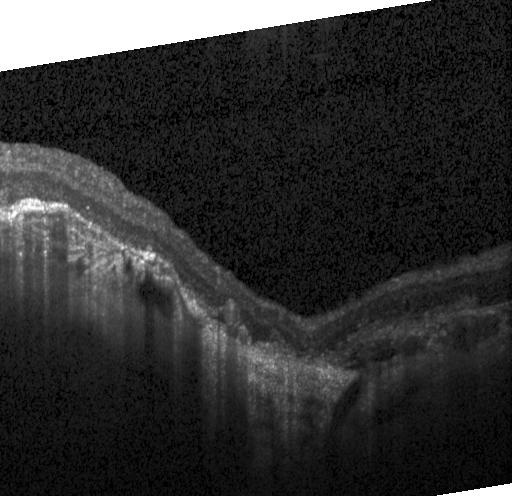
Optical coherence tomography B-scan. Spectral-domain OCT. This B-scan demonstrates a choroidal neovascular membrane.